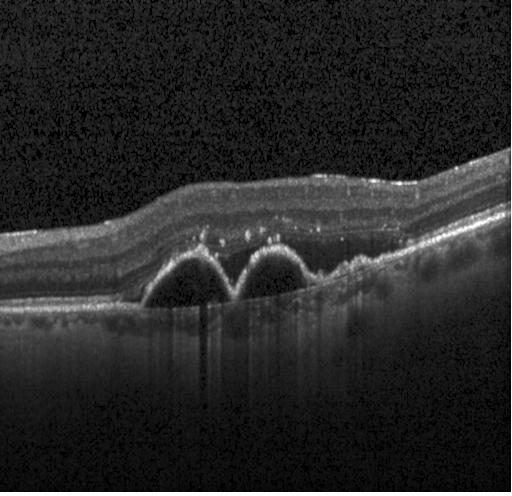 Optical coherence tomography B-scan; SD-OCT; horizontal scan through the fovea; acquired on a Heidelberg Spectralis.
The scan shows choroidal neovascularization (CNV).